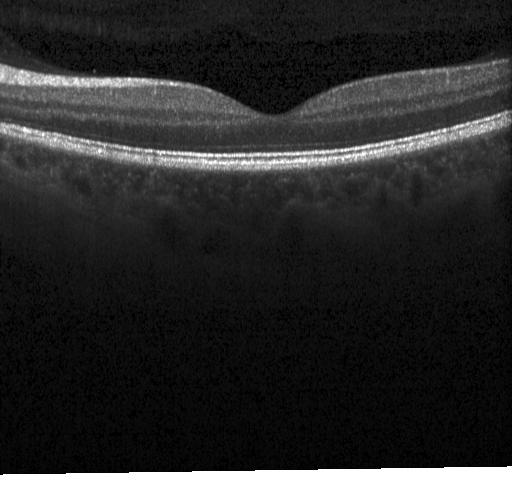

Impression: neither choroidal neovascularization, diabetic macular edema, nor drusen.